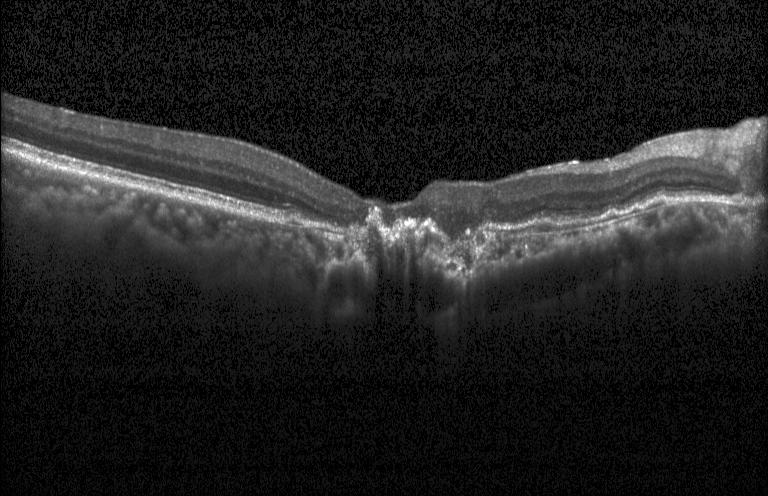
Retinal OCT B-scan, spectral-domain OCT, horizontal scan through the fovea — Assessment: choroidal neovascularization (CNV).